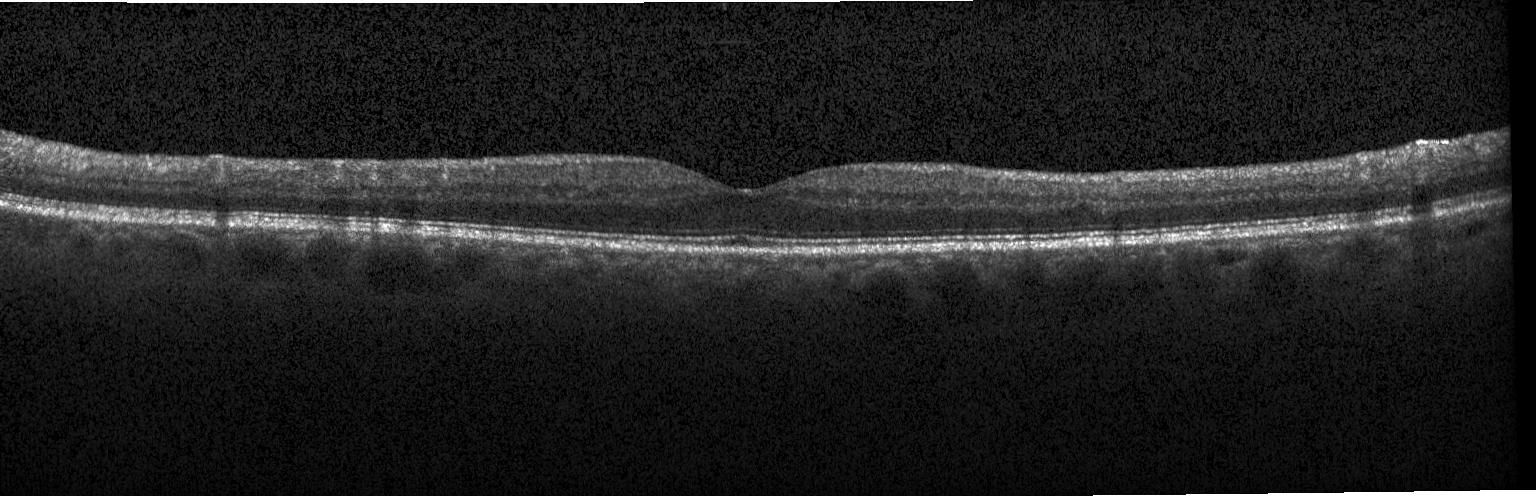 Heidelberg Spectralis OCT system; retinal OCT cross-section; SD-OCT — This B-scan demonstrates neither CNV, DME, nor drusen.